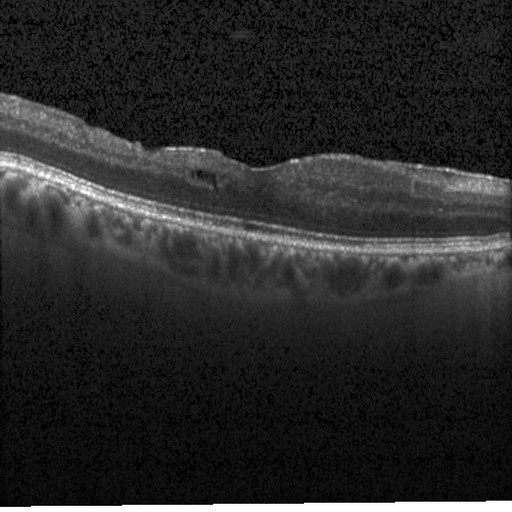
Spectral-domain optical coherence tomography. Retinal OCT B-scan — Diabetic macular edema.